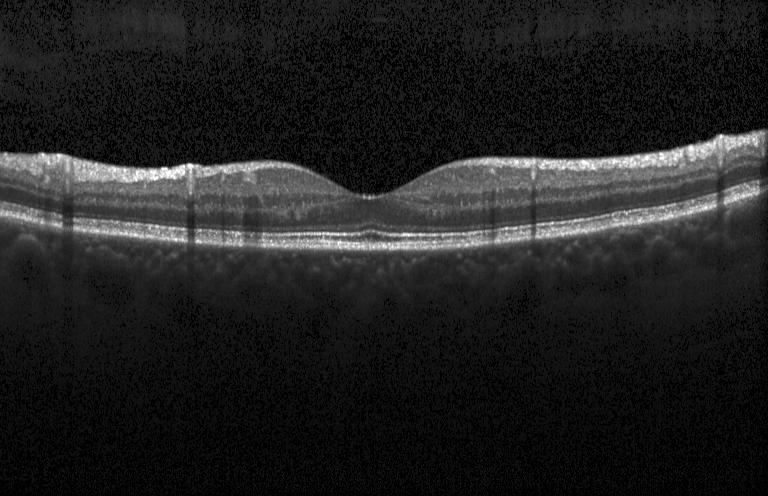
Optical coherence tomography B-scan, Heidelberg Spectralis OCT system, spectral-domain optical coherence tomography — Finding: no evidence of CNV, DME, or drusen.